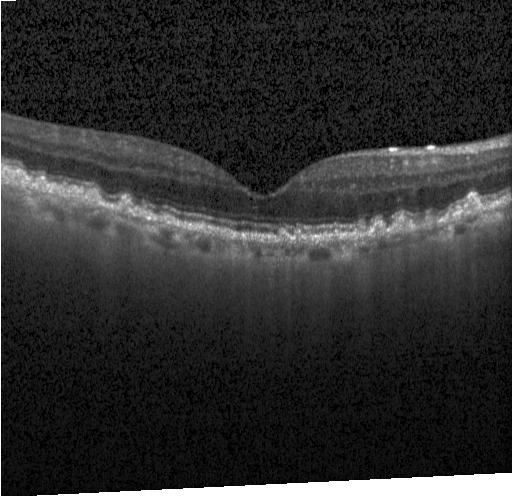 Fovea-centered, acquired on a Heidelberg Spectralis, optical coherence tomography scan, spectral-domain optical coherence tomography.
OCT finding: sub-RPE drusenoid deposits.